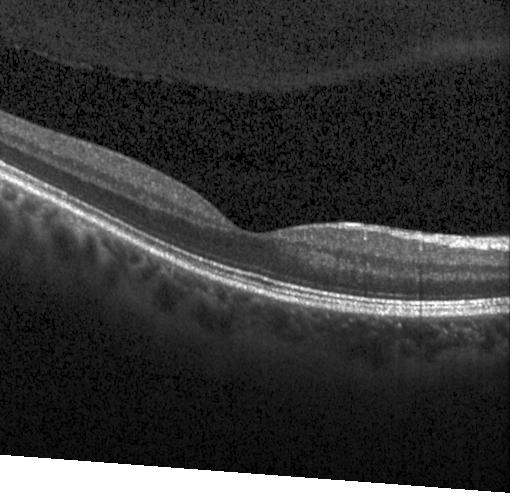
OCT B-scan. Assessment: no choroidal neovascularization, diabetic macular edema, or drusen.